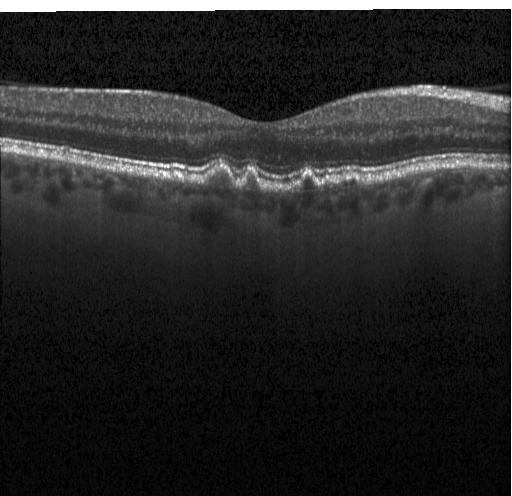
Retinal OCT B-scan.
Diagnosis: multiple drusen.